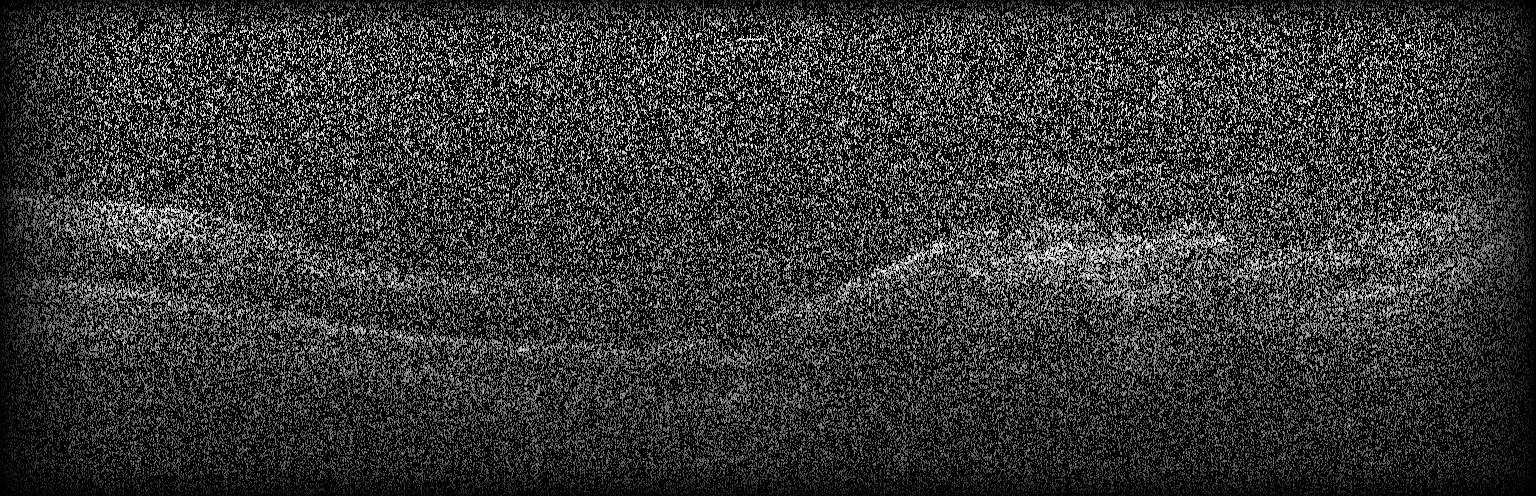
Retinal OCT B-scan — Impression: a choroidal neovascular membrane.